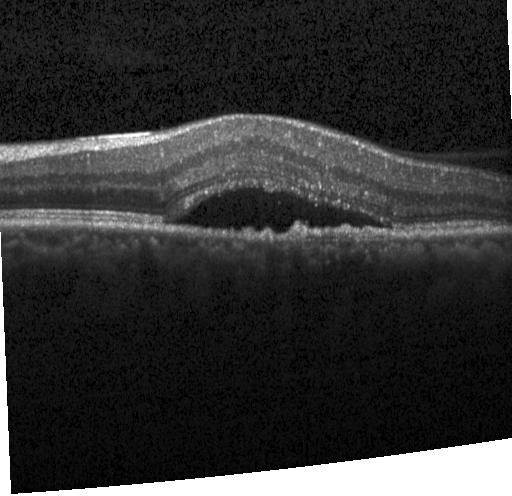

Spectral-domain optical coherence tomography · optical coherence tomography B-scan · Heidelberg Spectralis
Impression: a choroidal neovascular membrane.